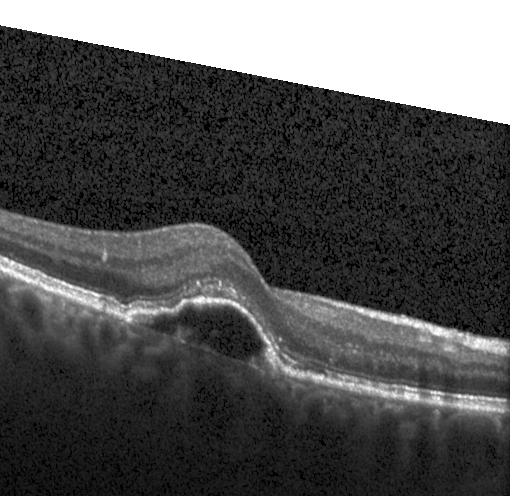
Centered on the fovea; OCT line scan; Heidelberg Spectralis — Dx: choroidal neovascularization (CNV).